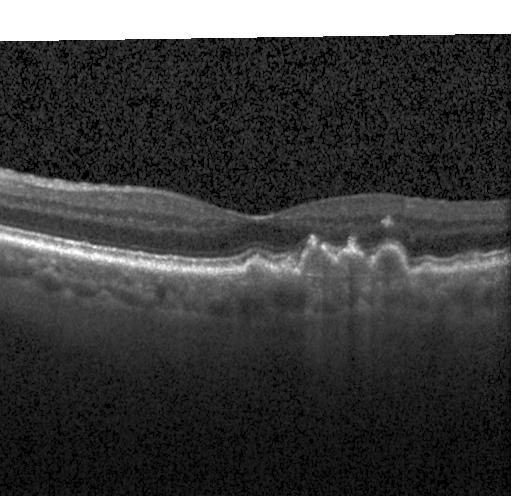
Optical coherence tomography scan; macular scan. Impression: sub-RPE drusenoid deposits.